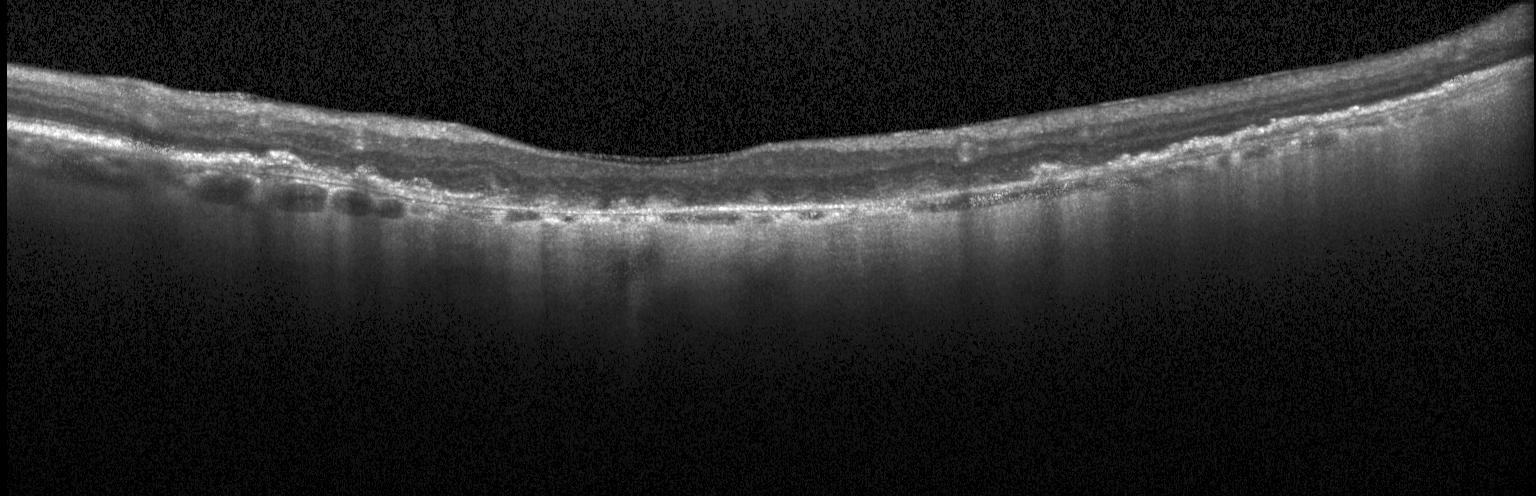

Diagnosis: choroidal neovascularization.